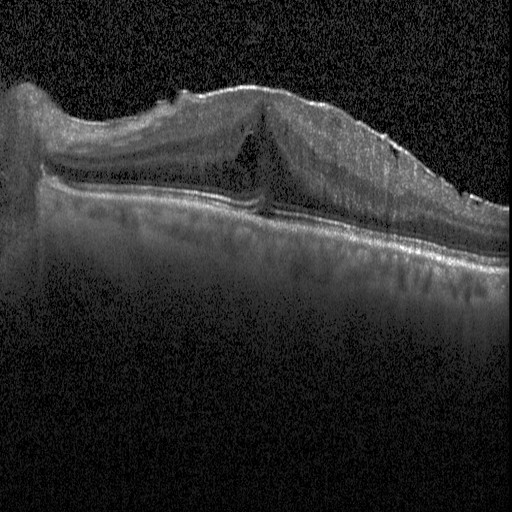

Retinal OCT B-scan. SD-OCT.
Finding: diabetic macular edema.